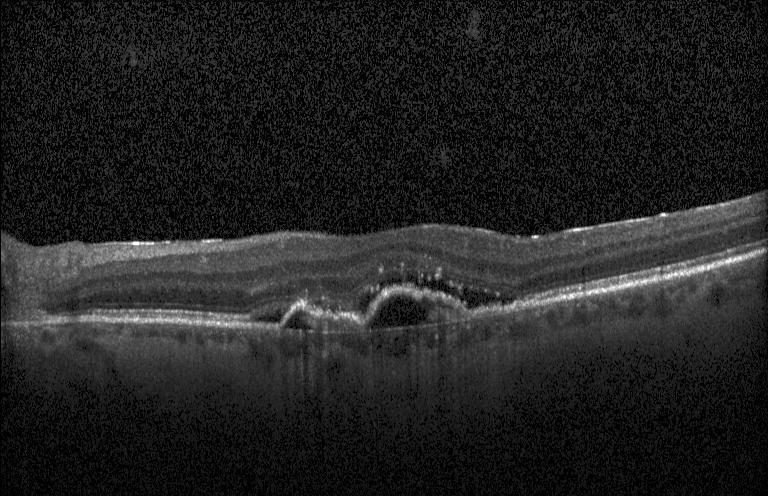 OCT finding: choroidal neovascularization (CNV).